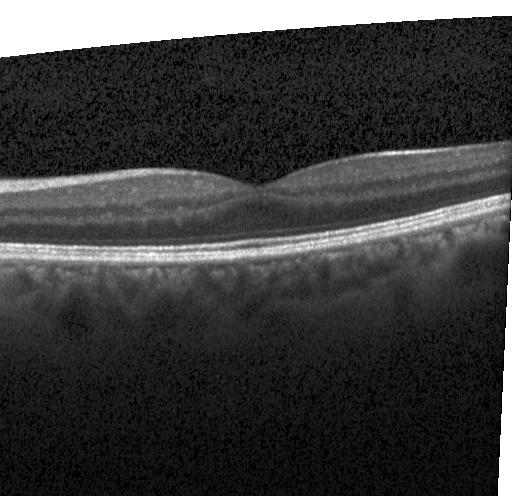 Assessment: no evidence of CNV, DME, or drusen.